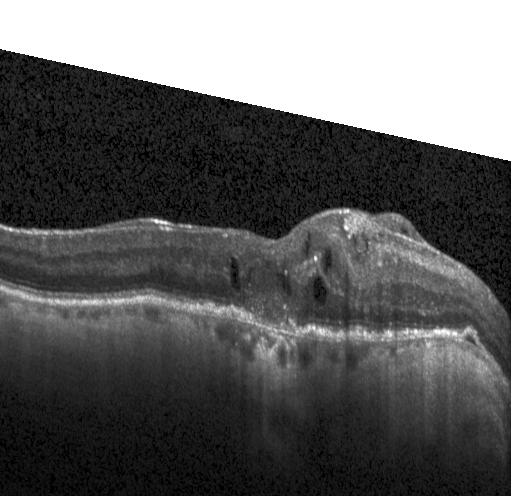 Macular OCT demonstrating choroidal neovascularization.